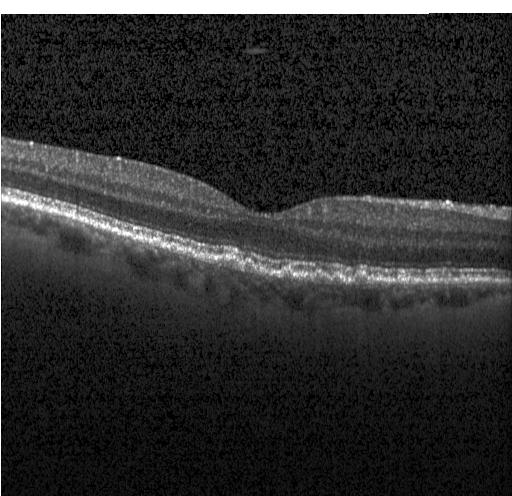 Drusen.